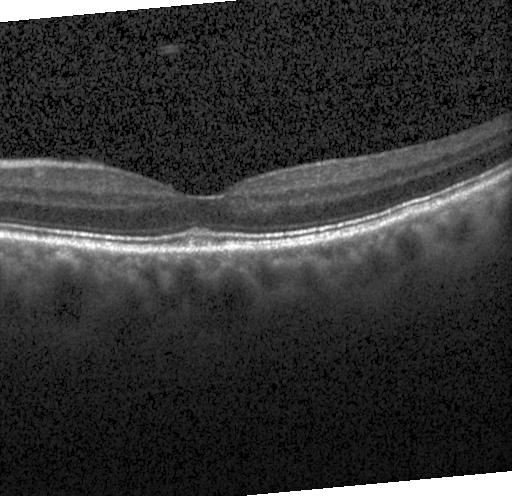 Optical coherence tomography B-scan. Acquired on a Heidelberg Spectralis — Finding: no evidence of CNV, DME, or drusen.